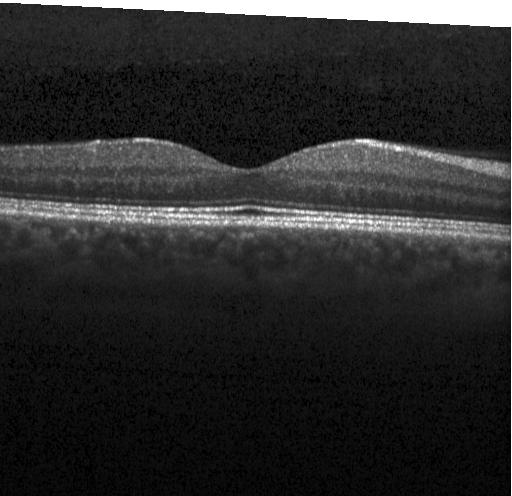
Optical coherence tomography B-scan
Assessment: no choroidal neovascularization, no diabetic macular edema, and no drusen.